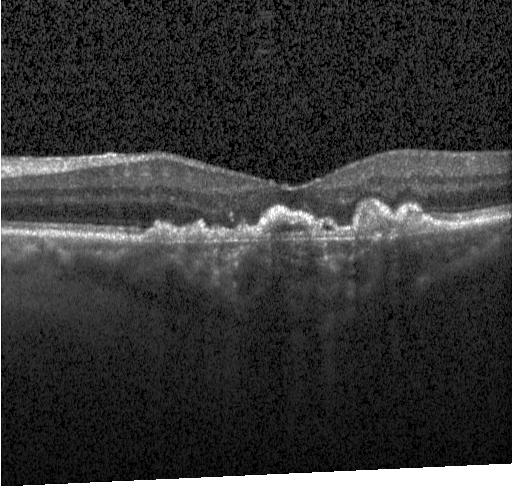 Macular OCT demonstrating a choroidal neovascular membrane.